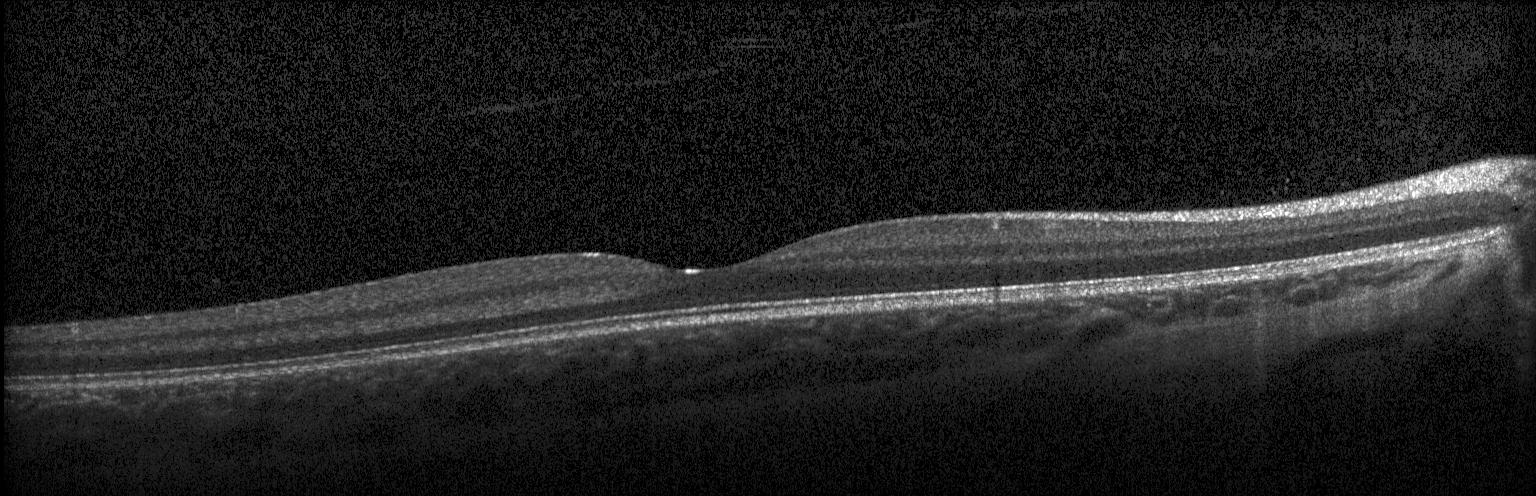

The scan shows neither CNV, DME, nor drusen.